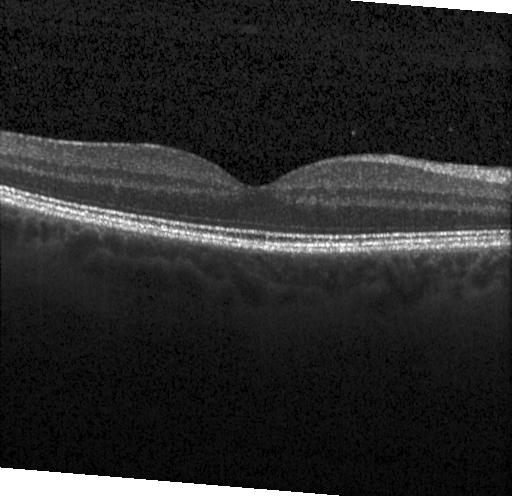 Macular OCT demonstrating no choroidal neovascularization, no diabetic macular edema, and no drusen.